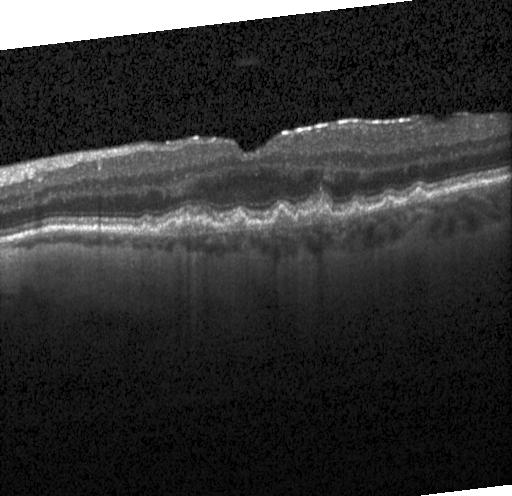

Optical coherence tomography scan.
Dx: sub-RPE drusenoid deposits.